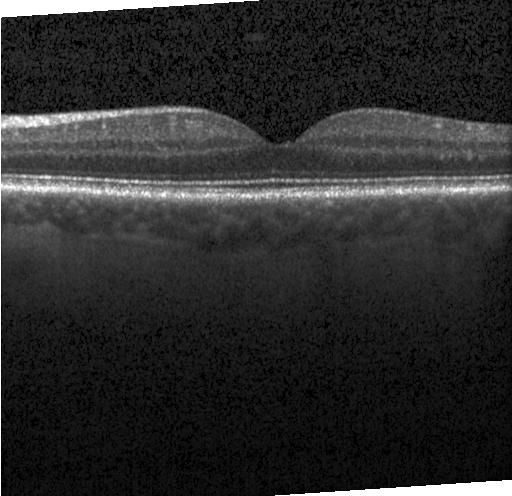

Dx: no choroidal neovascularization, diabetic macular edema, or drusen.